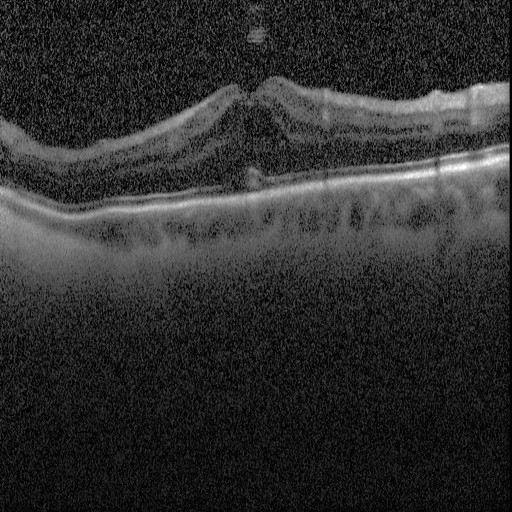

OCT B-scan — Diabetic macular edema (DME).